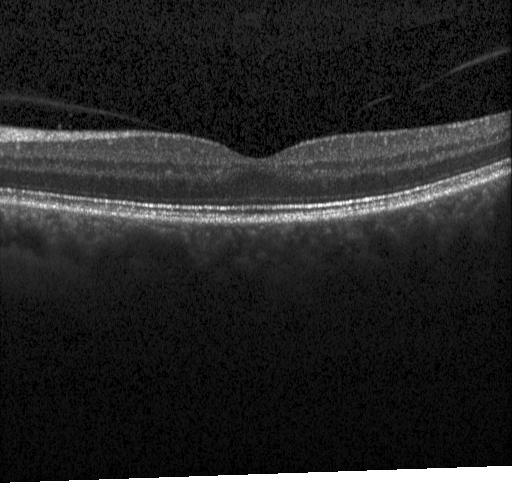
Optical coherence tomography B-scan. Heidelberg Spectralis OCT system. Macular scan
Assessment: no evidence of CNV, DME, or drusen.